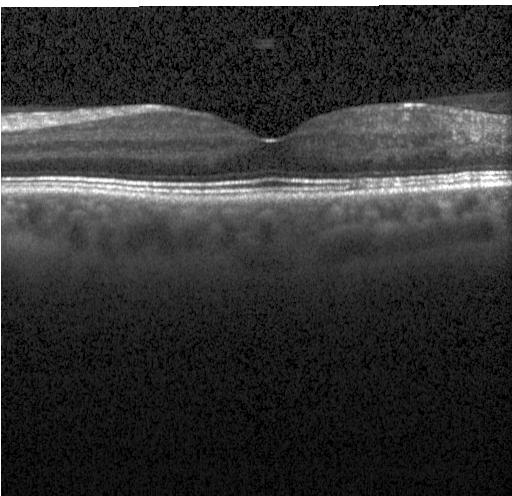 The scan shows no evidence of choroidal neovascularization, diabetic macular edema, or drusen.